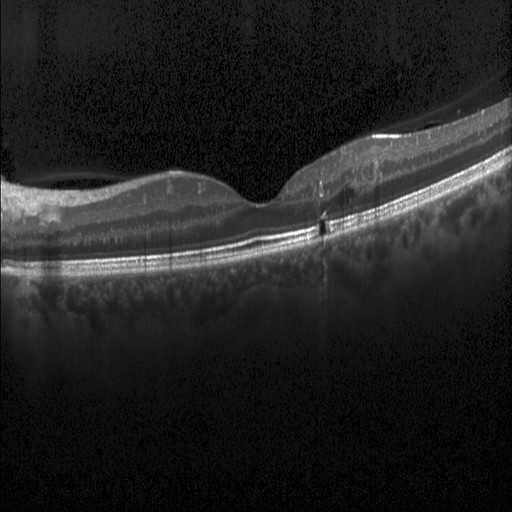
The scan shows diabetic macular edema (DME).